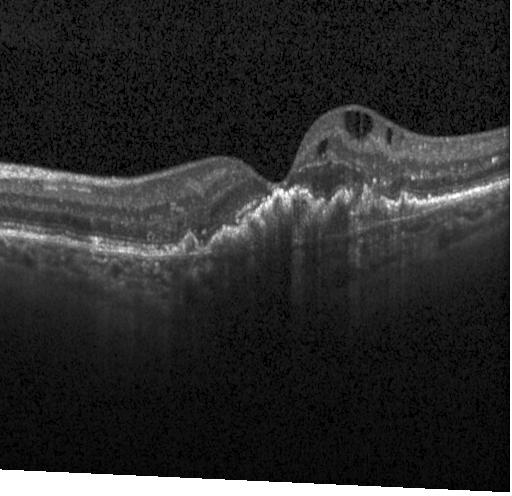
The scan shows a choroidal neovascular membrane.